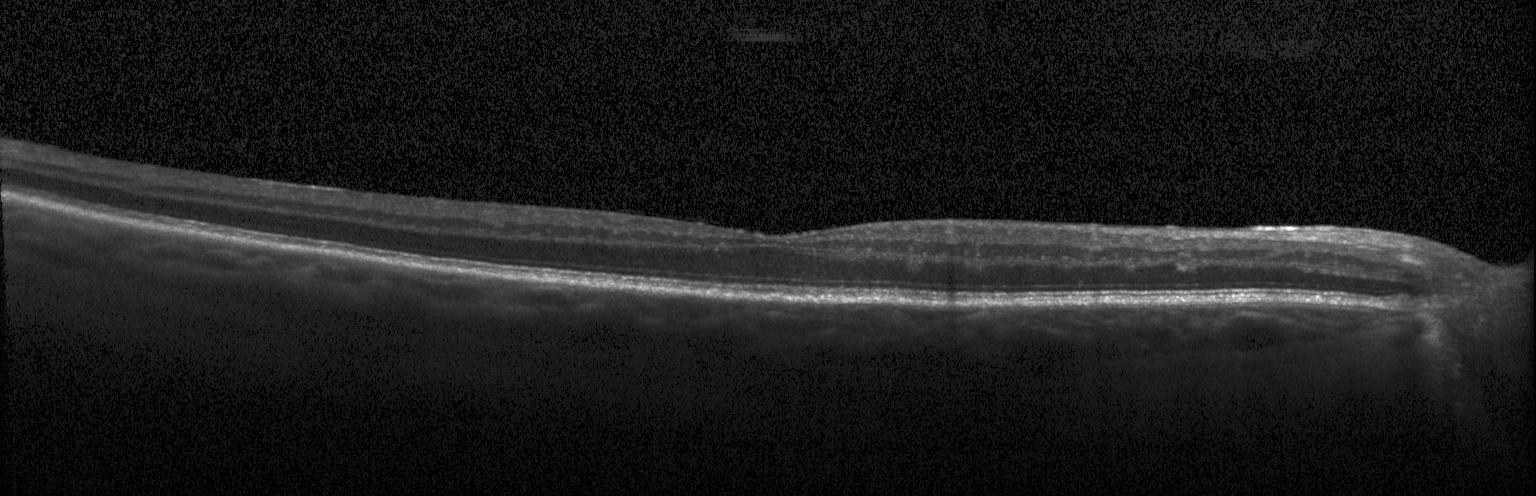 Retinal OCT B-scan; macular scan; spectral-domain optical coherence tomography; instrument: Heidelberg Spectralis
Finding: no evidence of choroidal neovascularization, diabetic macular edema, or drusen.